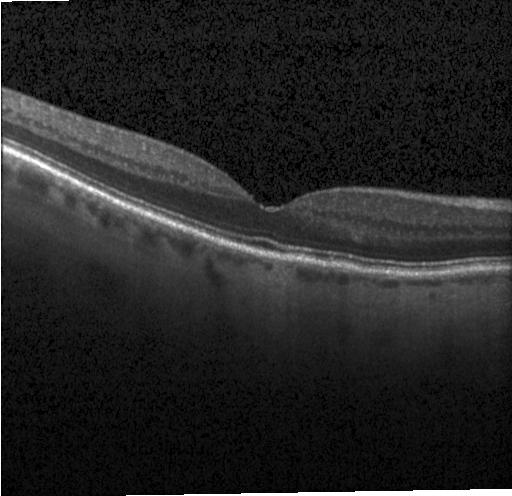
Macular OCT demonstrating neither choroidal neovascularization, diabetic macular edema, nor drusen.